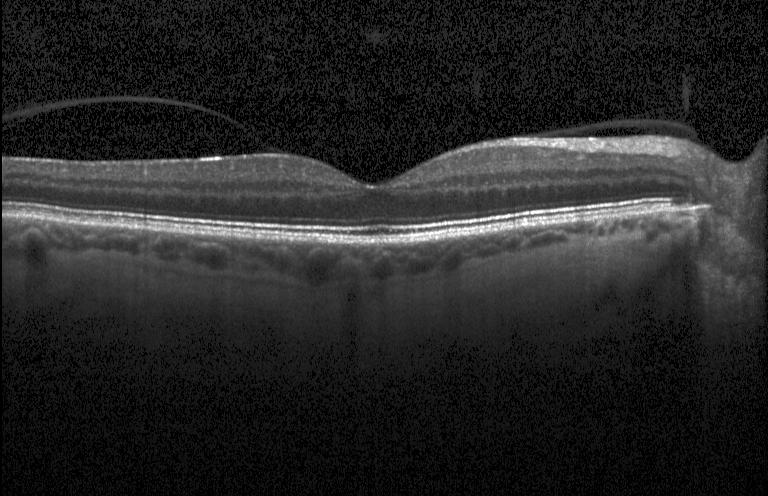 OCT line scan, through the macula, Heidelberg Spectralis, SD-OCT
Impression: no choroidal neovascularization, diabetic macular edema, or drusen.